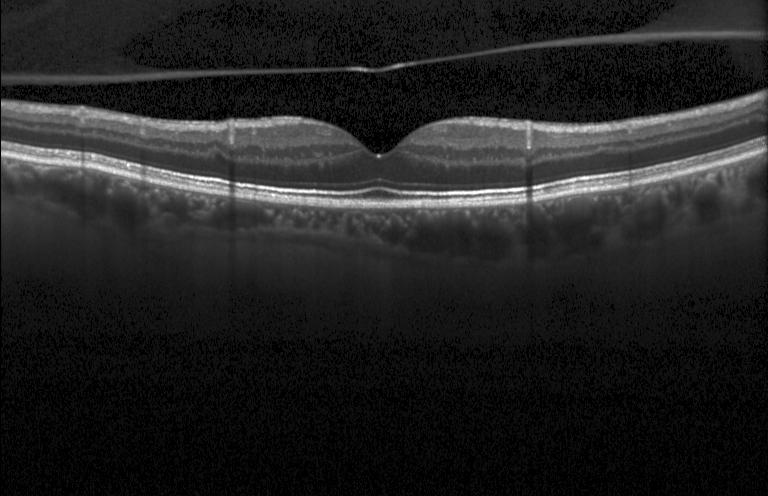 SD-OCT; optical coherence tomography B-scan.
Dx: no choroidal neovascularization, no diabetic macular edema, and no drusen.